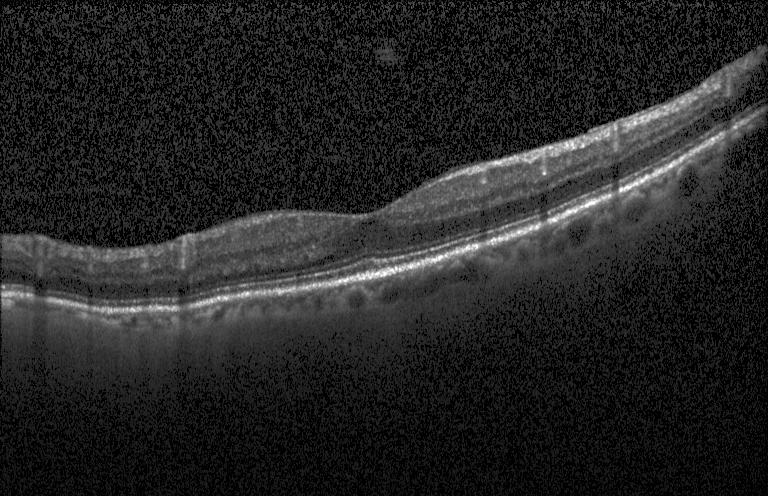
Optical coherence tomography B-scan. Diagnosis: no evidence of choroidal neovascularization, diabetic macular edema, or drusen.